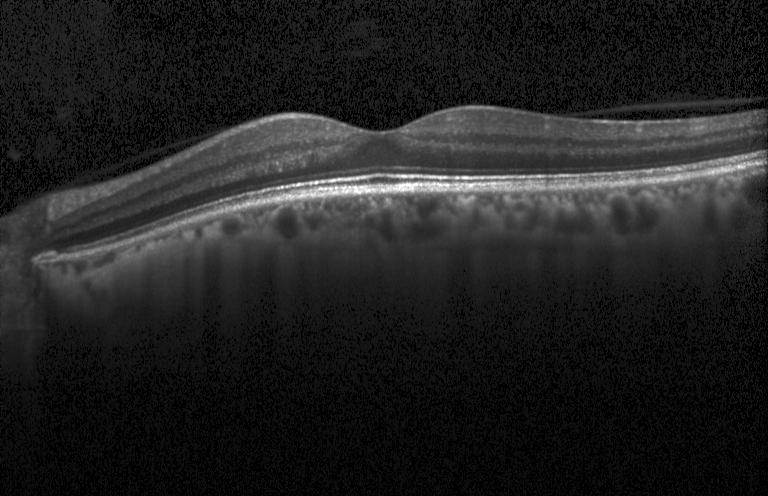
Optical coherence tomography scan — Diagnosis: neither CNV, DME, nor drusen.